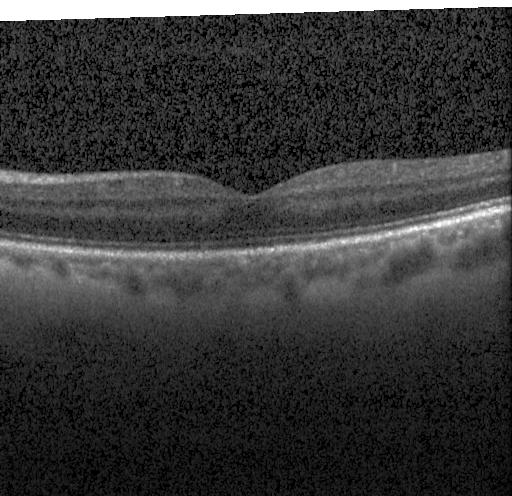 Fovea-centered. Retinal OCT cross-section. Spectral-domain OCT — Impression: no choroidal neovascularization, no diabetic macular edema, and no drusen.